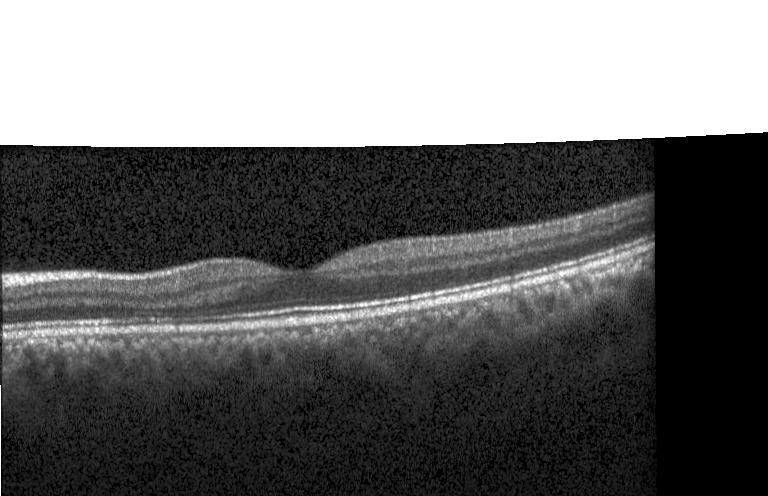 Spectral-domain optical coherence tomography; optical coherence tomography B-scan; horizontal scan through the fovea
The scan shows neither choroidal neovascularization, diabetic macular edema, nor drusen.